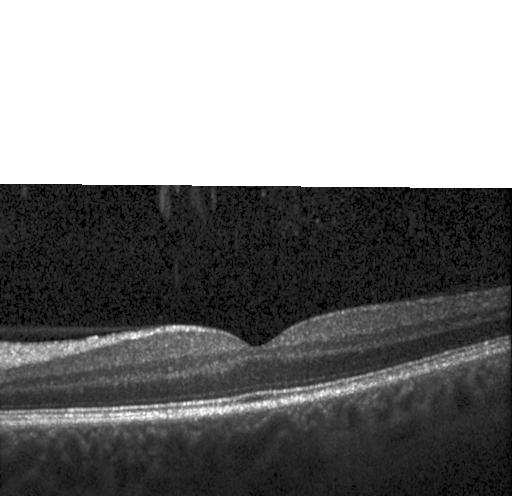
Optical coherence tomography scan.
Finding: no choroidal neovascularization, no diabetic macular edema, and no drusen.